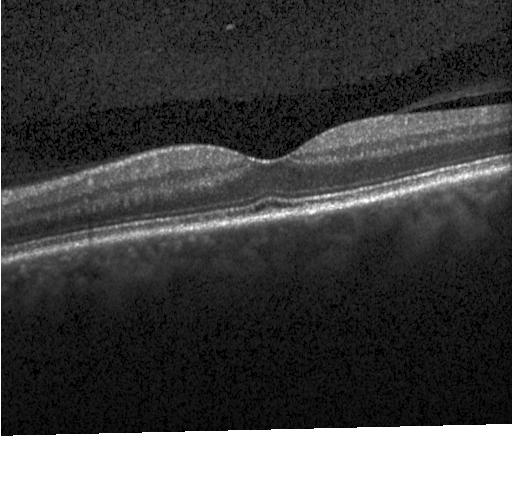

Optical coherence tomography scan · instrument: Heidelberg Spectralis · horizontal scan through the fovea · spectral-domain OCT
Diagnosis: no evidence of choroidal neovascularization, diabetic macular edema, or drusen.